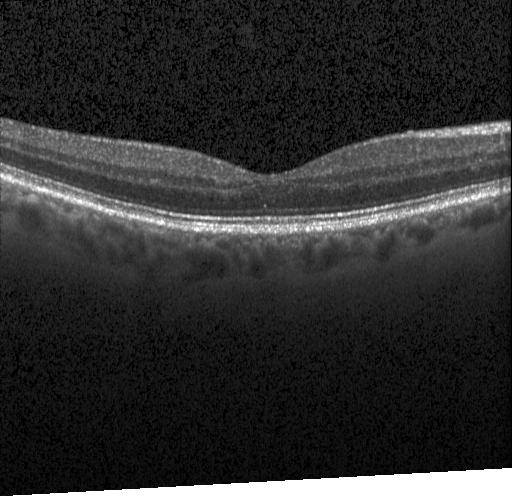
Horizontal scan through the fovea; acquired on a Heidelberg Spectralis; OCT B-scan; spectral-domain OCT.
Diagnosis: no choroidal neovascularization, diabetic macular edema, or drusen.